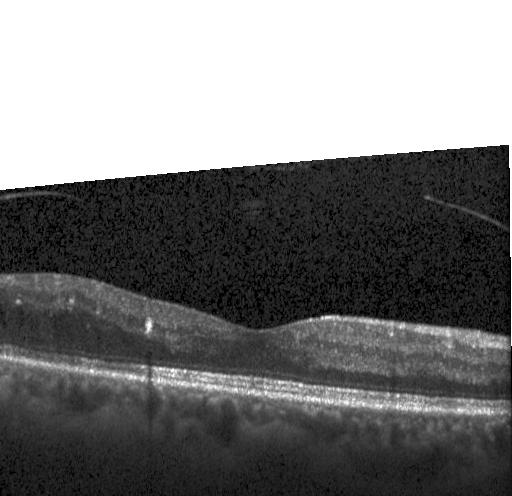
OCT B-scan · acquired on a Heidelberg Spectralis · spectral-domain optical coherence tomography. Assessment: diabetic macular edema.